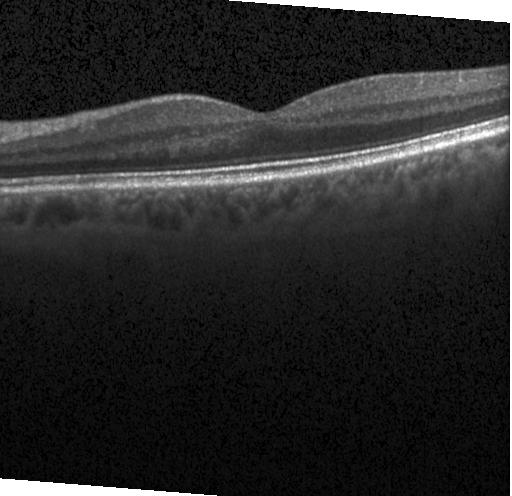 Impression: no choroidal neovascularization, no diabetic macular edema, and no drusen.